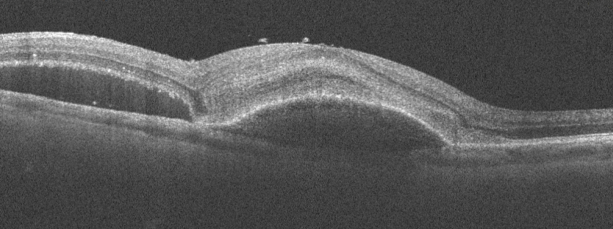
OCT B-scan. Acquired on an Optovue Avanti RTVue XR — Impression: AMD.